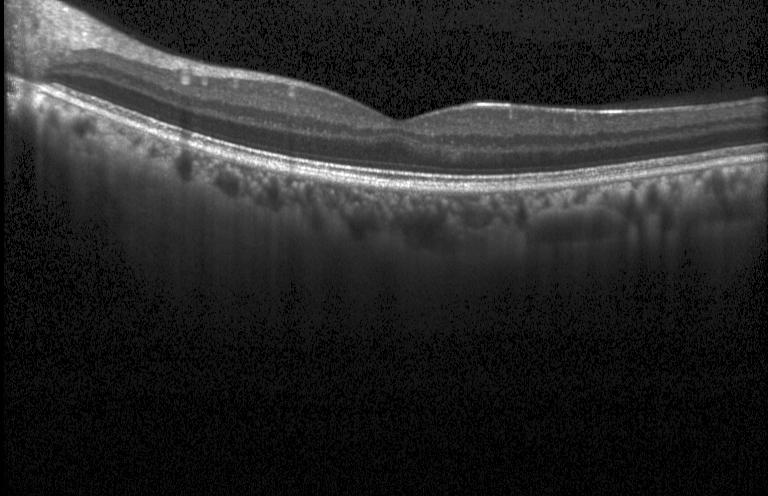

OCT B-scan.
Finding: no choroidal neovascularization, diabetic macular edema, or drusen.